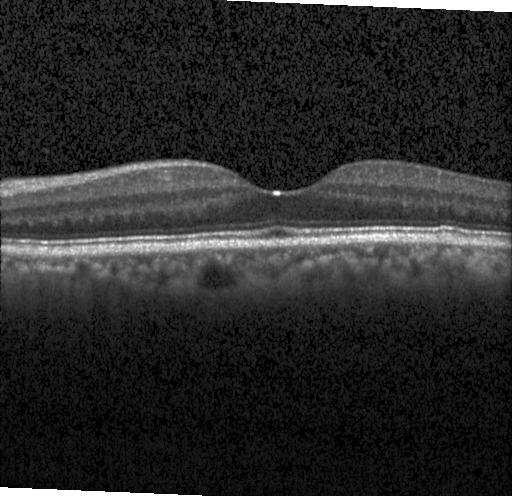 Heidelberg Spectralis, retinal OCT B-scan, centered on the fovea, spectral-domain OCT — Impression: no choroidal neovascularization, no diabetic macular edema, and no drusen.